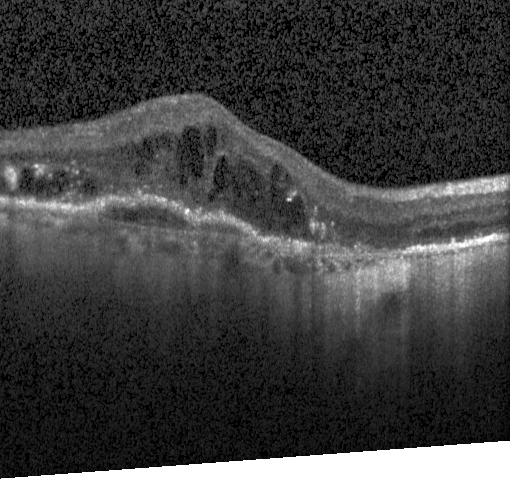 Retinal OCT cross-section
Dx: choroidal neovascularization (CNV).